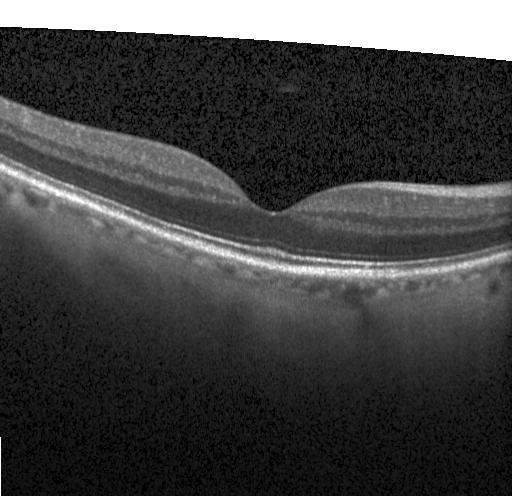 SD-OCT; OCT line scan.
Impression: no choroidal neovascularization, diabetic macular edema, or drusen.